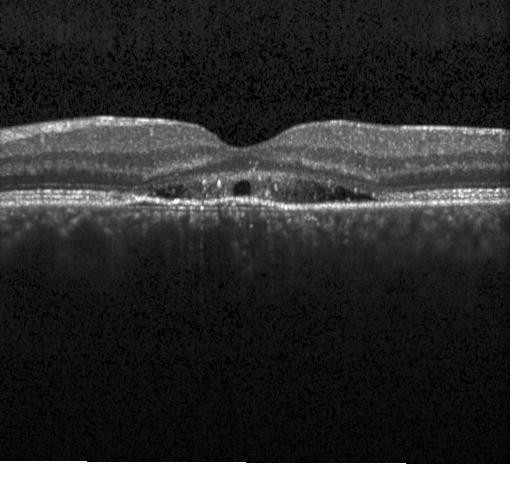

Retinal OCT cross-section. Macular scan. Acquired on a Heidelberg Spectralis
Diagnosis: a choroidal neovascular membrane.